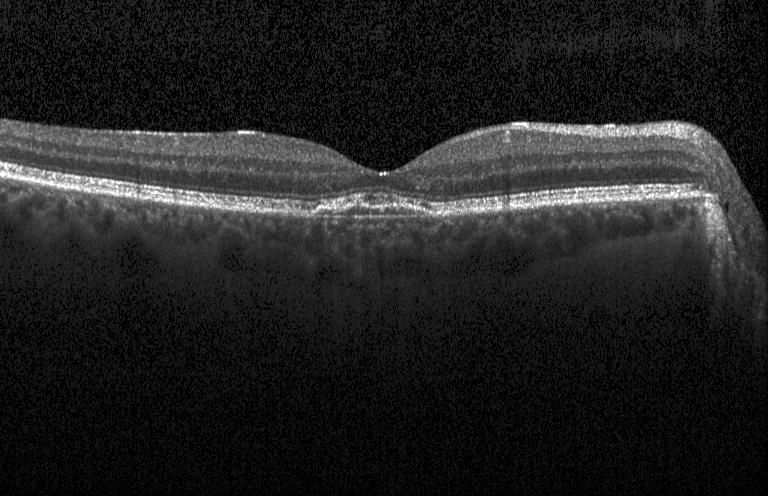
Finding: a choroidal neovascular membrane.